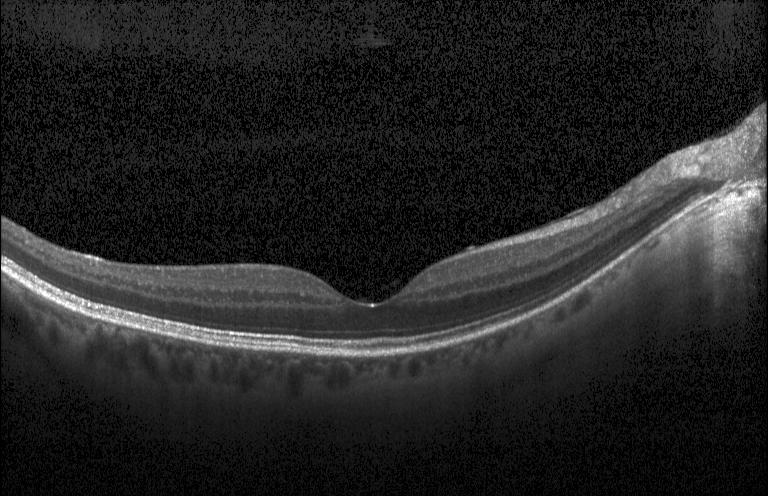

Optical coherence tomography B-scan, SD-OCT
Impression: neither choroidal neovascularization, diabetic macular edema, nor drusen.